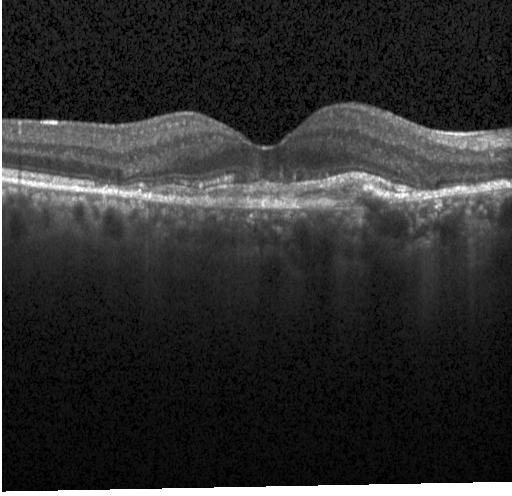 Acquired on a Heidelberg Spectralis · horizontal scan through the fovea · retinal OCT B-scan. Macular OCT: choroidal neovascularization.